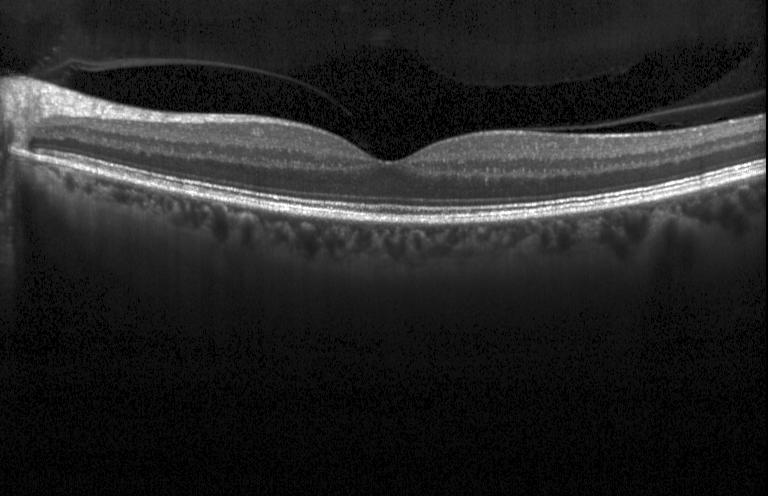 Dx: no choroidal neovascularization, diabetic macular edema, or drusen.